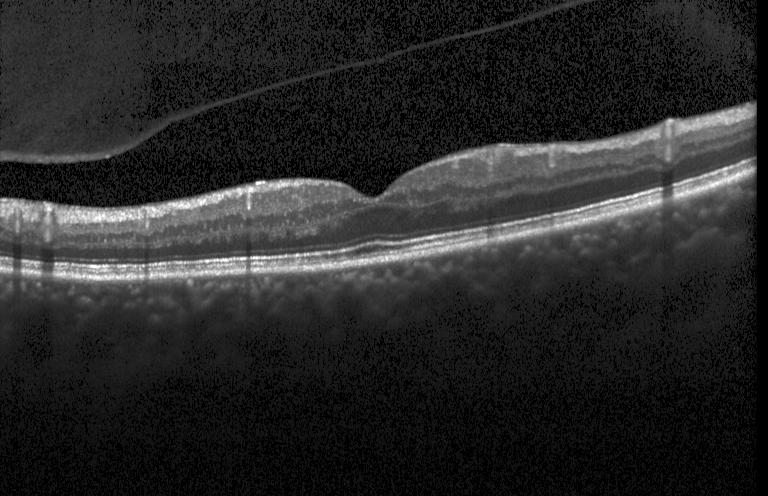 OCT line scan — Assessment: no CNV, no DME, and no drusen.